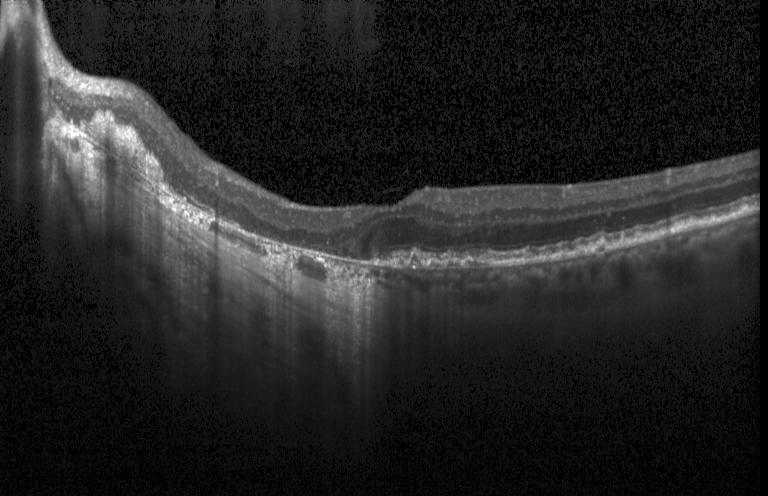

OCT B-scan. Impression: a choroidal neovascular membrane.